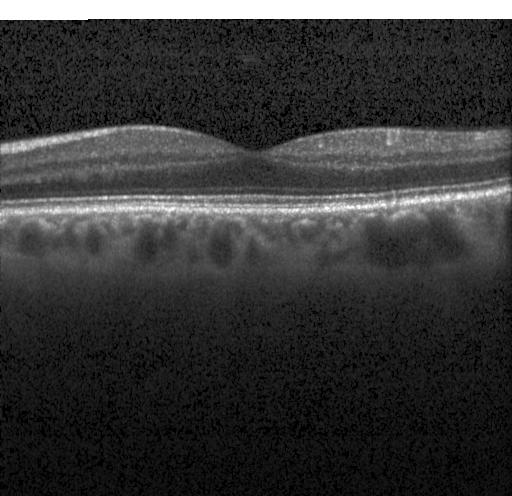

Spectral-domain optical coherence tomography, OCT line scan — Finding: no choroidal neovascularization, diabetic macular edema, or drusen.